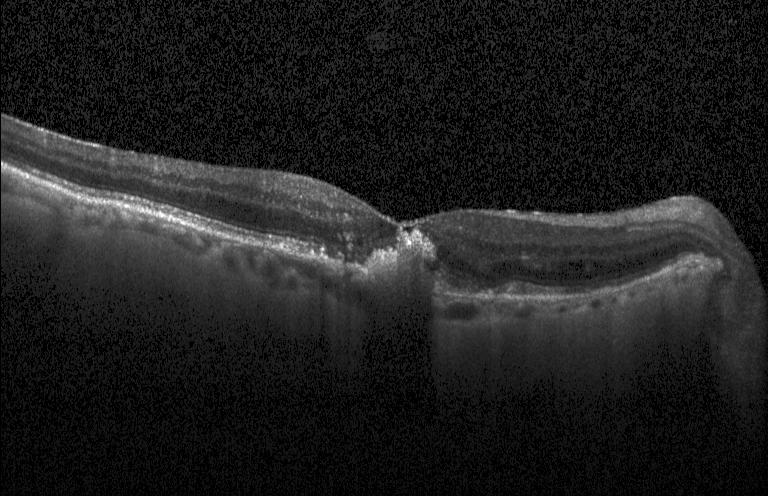
OCT line scan
Macular OCT: CNV.